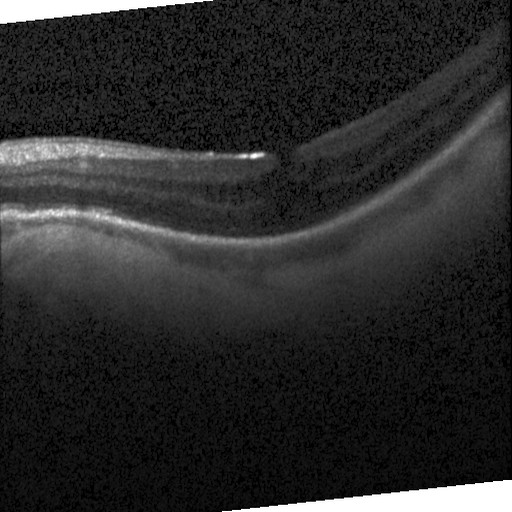 Instrument: Heidelberg Spectralis; optical coherence tomography scan
Diagnosis: diabetic macular edema.